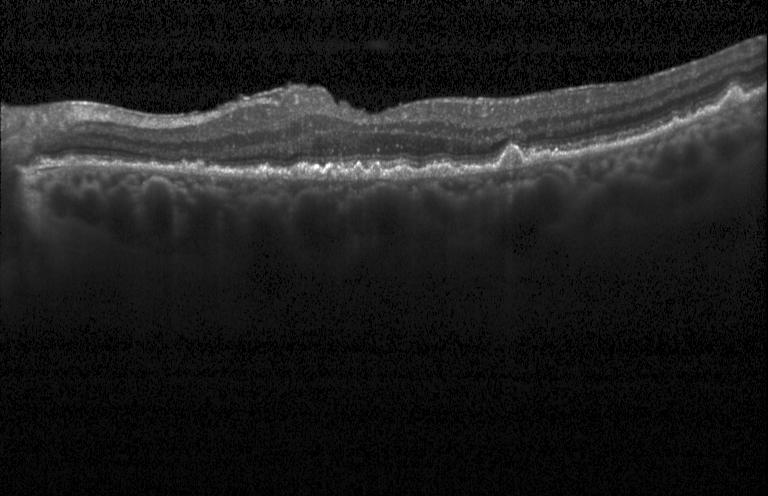 SD-OCT; retinal OCT cross-section; macular scan.
Impression: drusen.